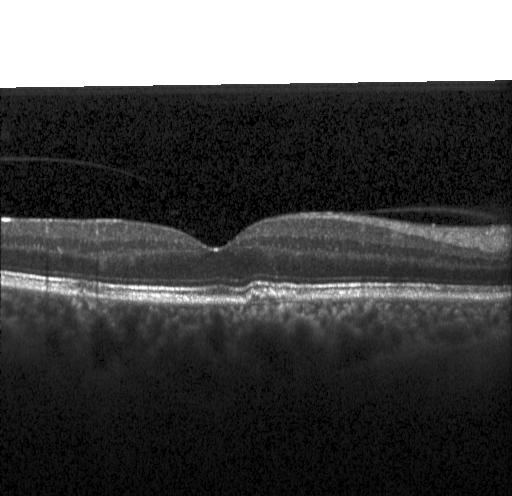

Optical coherence tomography scan — Macular OCT: sub-RPE drusenoid deposits.